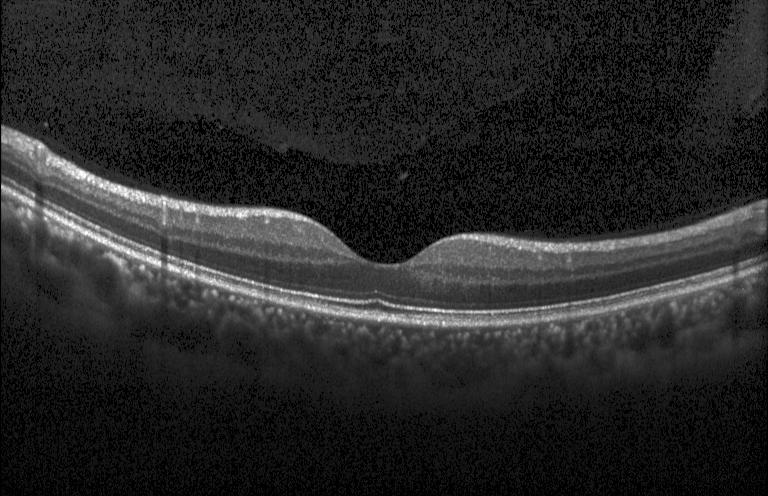
Macular scan, SD-OCT, OCT line scan. Macular OCT: no choroidal neovascularization, diabetic macular edema, or drusen.